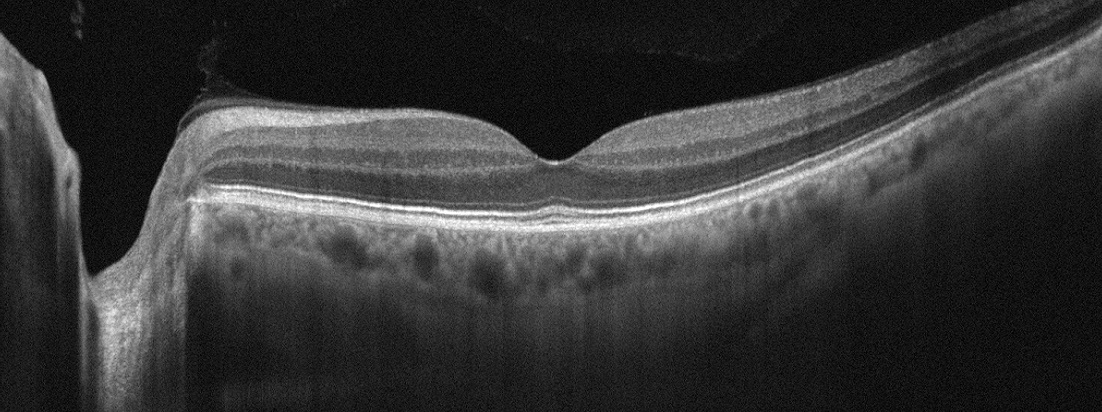 OCT B-scan · through the macula · Optovue Avanti RTVue XR.
Impression: absence of AMD, DME, ERM, RAO, RVO, and vitreomacular interface disease.